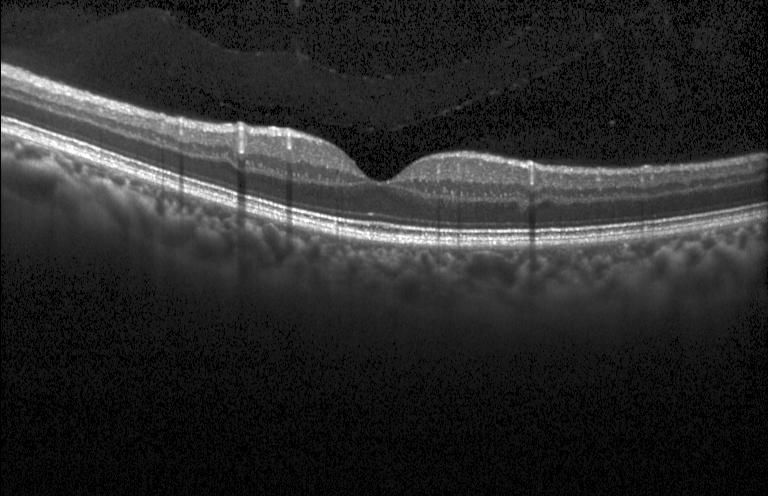

Assessment: no choroidal neovascularization, no diabetic macular edema, and no drusen.